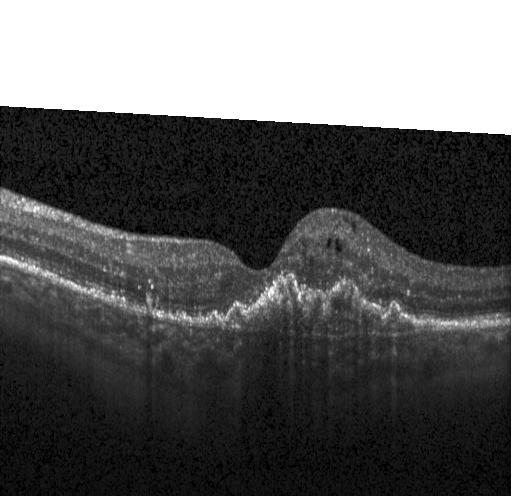
Spectral-domain optical coherence tomography, optical coherence tomography B-scan. Impression: CNV.